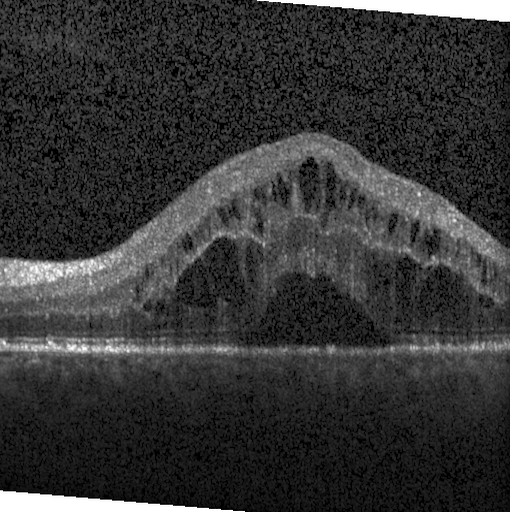 Finding: diabetic macular edema.